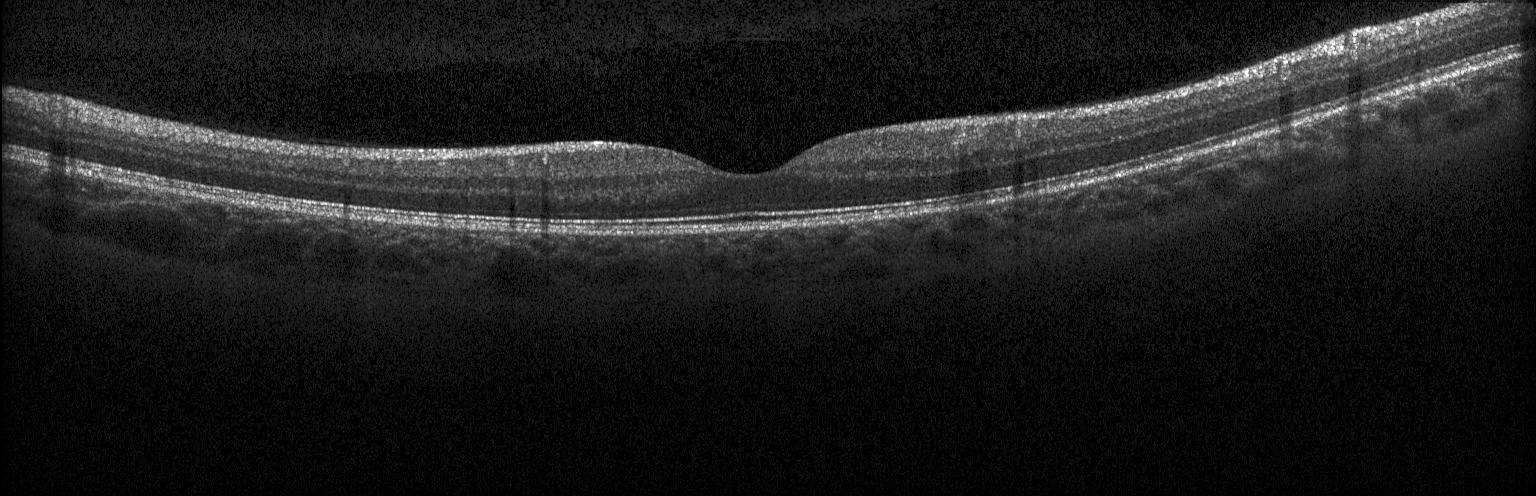
Optical coherence tomography scan · SD-OCT · Heidelberg Spectralis OCT system — The scan shows neither choroidal neovascularization, diabetic macular edema, nor drusen.